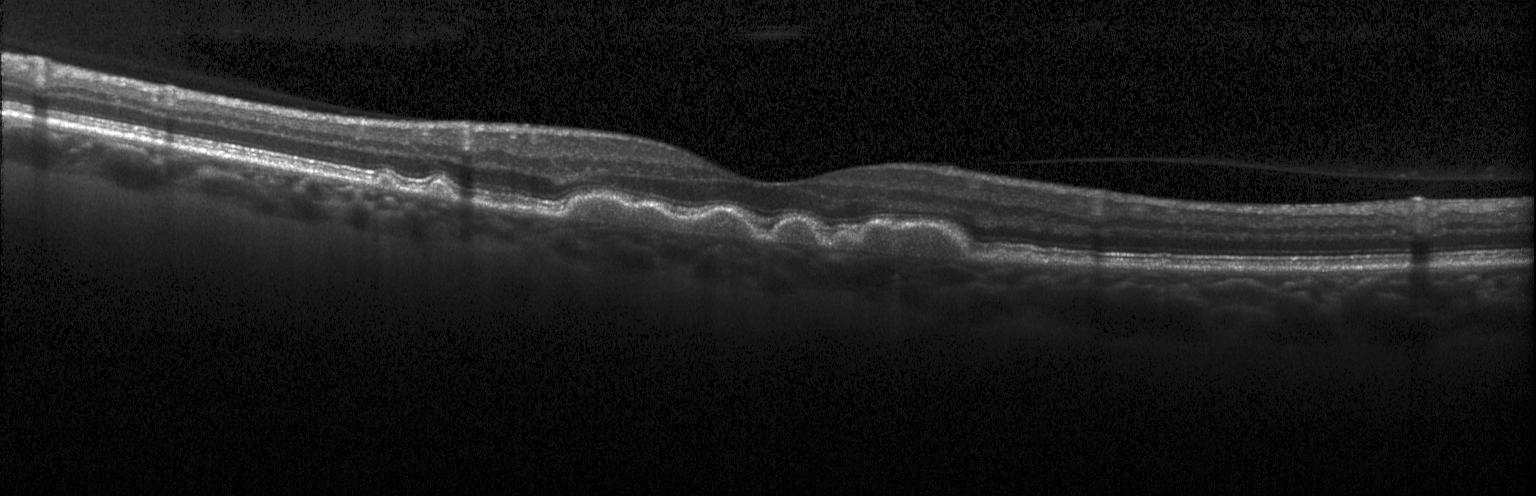
Impression: a choroidal neovascular membrane.